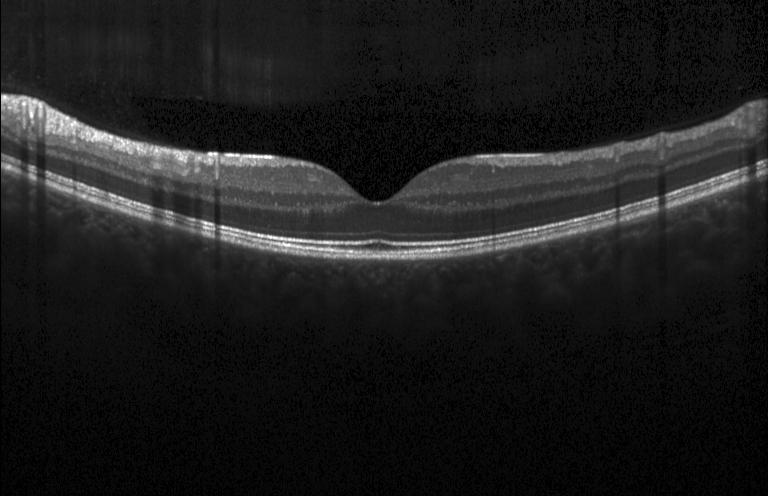
OCT B-scan. Heidelberg Spectralis. Through the macula. SD-OCT — Finding: no CNV, no DME, and no drusen.